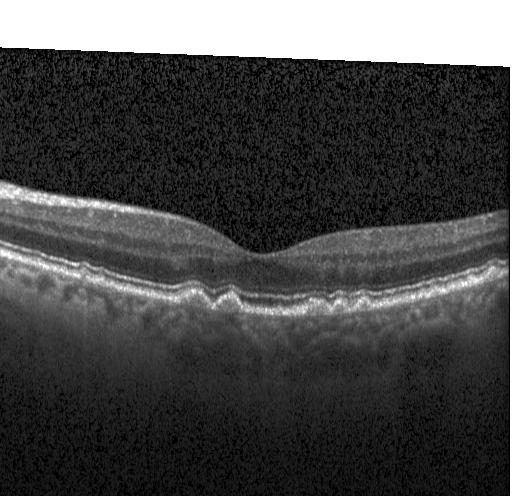

Centered on the fovea; retinal OCT cross-section — Impression: sub-RPE drusenoid deposits.